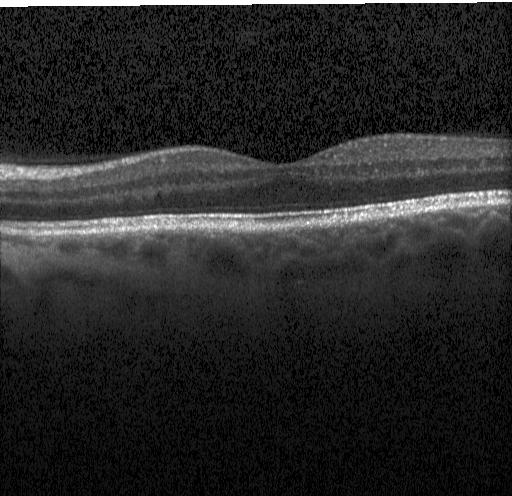

Instrument: Heidelberg Spectralis; optical coherence tomography scan; through the macula. Diagnosis: no choroidal neovascularization, no diabetic macular edema, and no drusen.